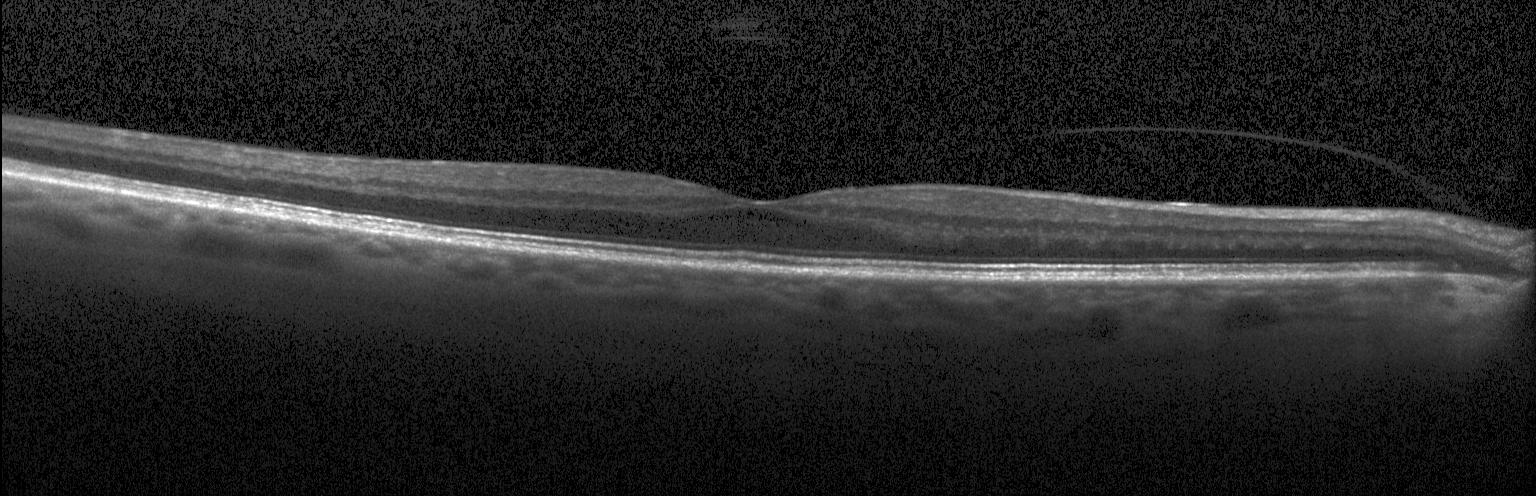

Heidelberg Spectralis OCT system, SD-OCT, OCT line scan, centered on the fovea
The scan shows no evidence of choroidal neovascularization, diabetic macular edema, or drusen.